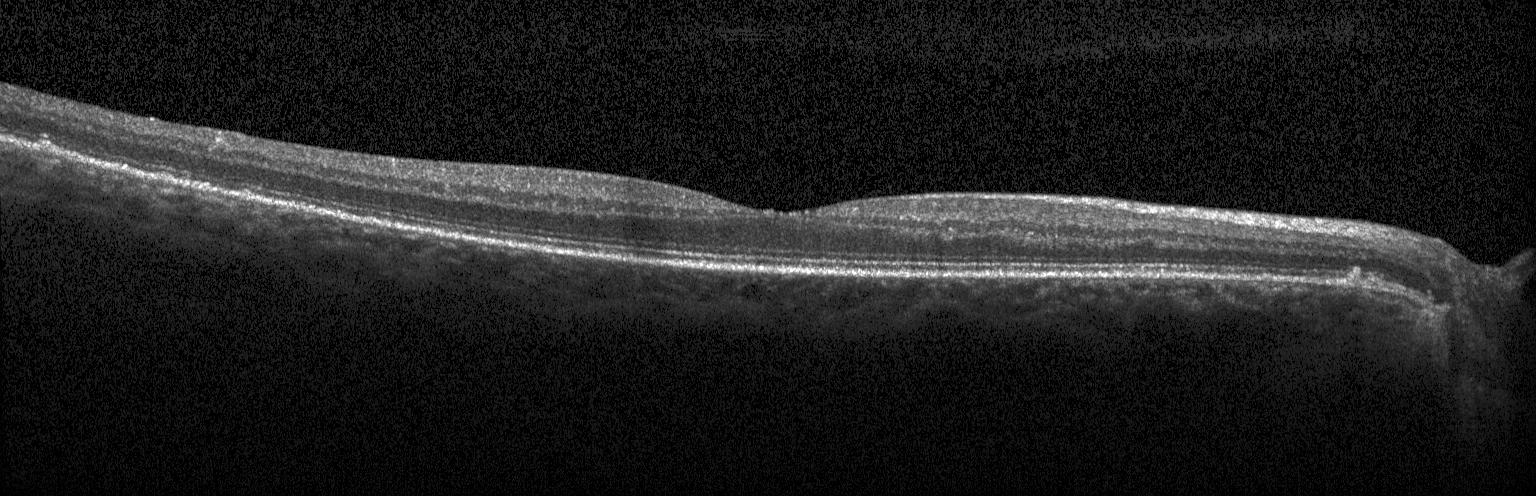
Optical coherence tomography scan · SD-OCT · Heidelberg Spectralis OCT system
Impression: neither choroidal neovascularization, diabetic macular edema, nor drusen.